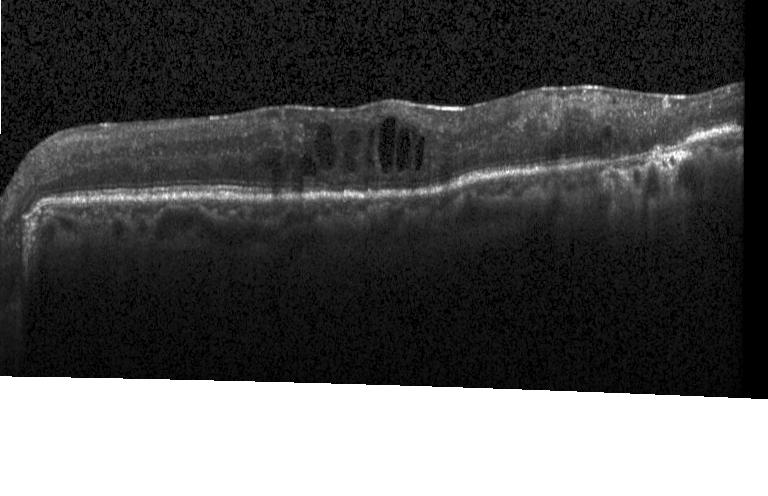
Spectral-domain OCT. Through the macula. Instrument: Heidelberg Spectralis. Optical coherence tomography B-scan.
Macular OCT: diabetic macular edema.